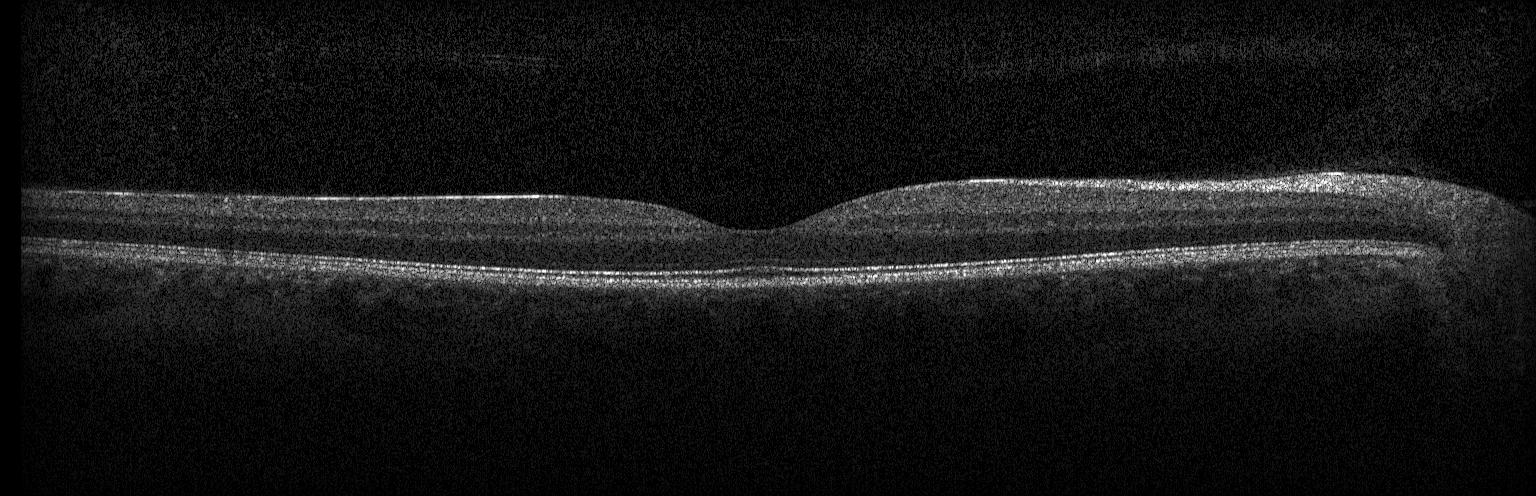

Retinal OCT B-scan
Assessment: neither choroidal neovascularization, diabetic macular edema, nor drusen.